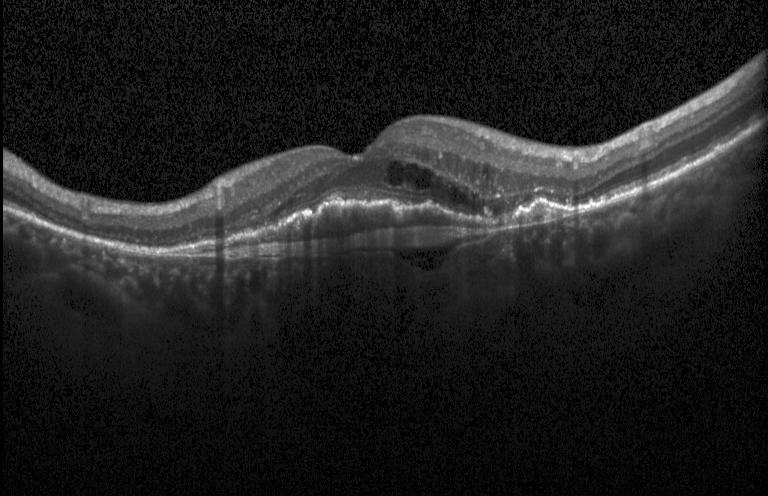

Heidelberg Spectralis OCT system. Spectral-domain optical coherence tomography. OCT B-scan — The scan shows a choroidal neovascular membrane.